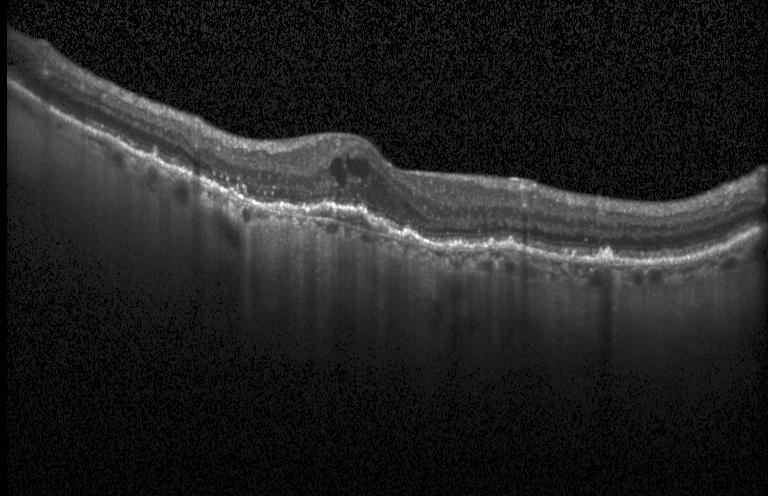

Diagnosis: a choroidal neovascular membrane.